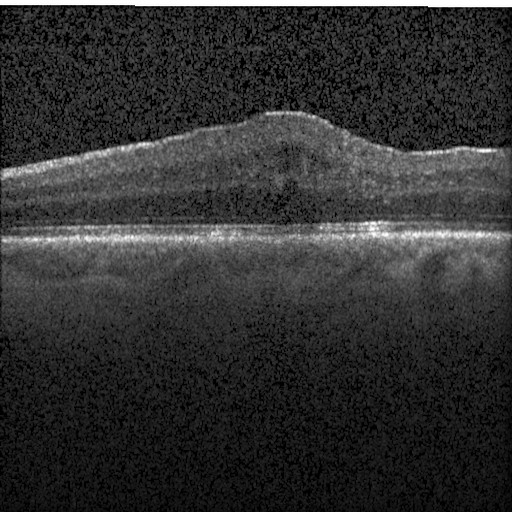 Macular OCT: diabetic macular edema.